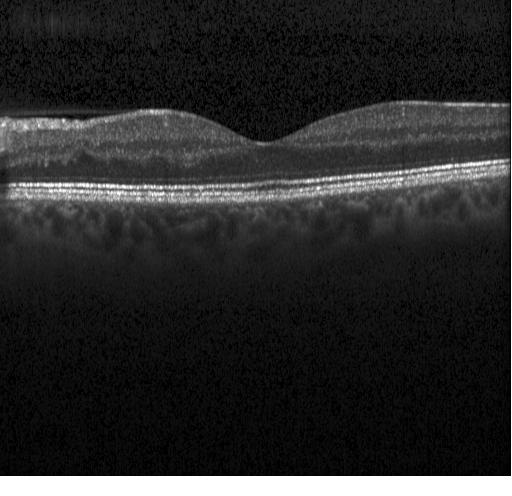
This B-scan demonstrates no CNV, no DME, and no drusen.